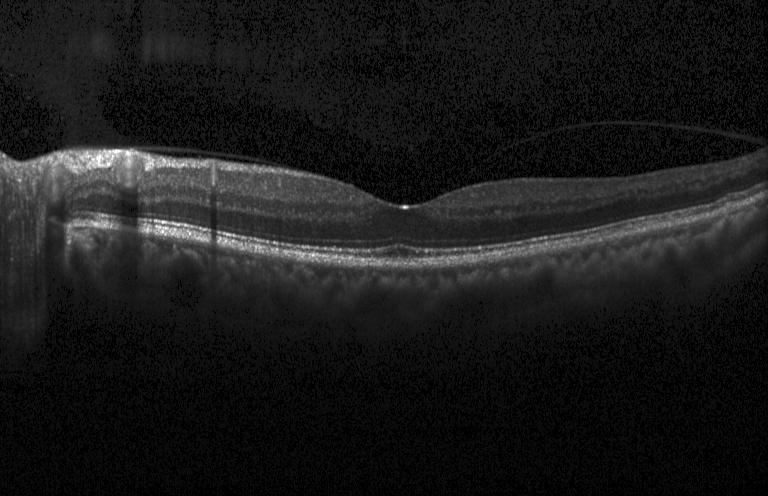
Impression: no choroidal neovascularization, no diabetic macular edema, and no drusen.